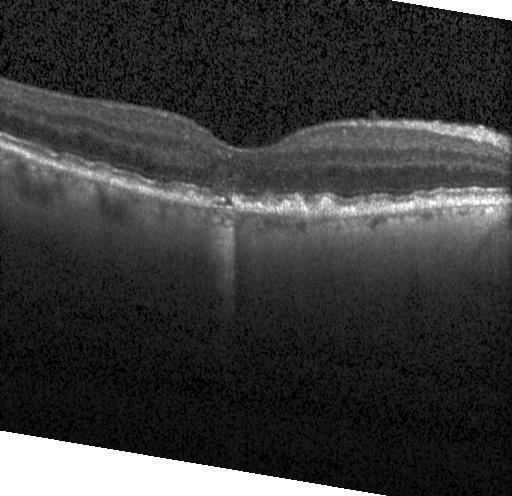 Instrument: Heidelberg Spectralis, spectral-domain OCT, retinal OCT B-scan.
Impression: multiple drusen.